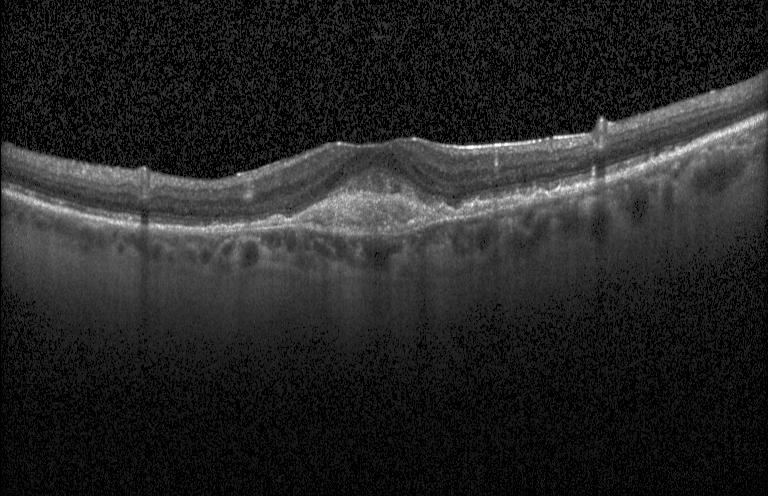

Instrument: Heidelberg Spectralis; optical coherence tomography scan; through the macula
Impression: CNV.